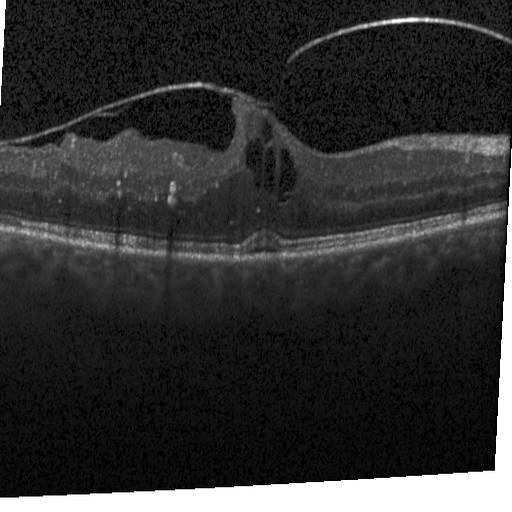
Diagnosis: DME.